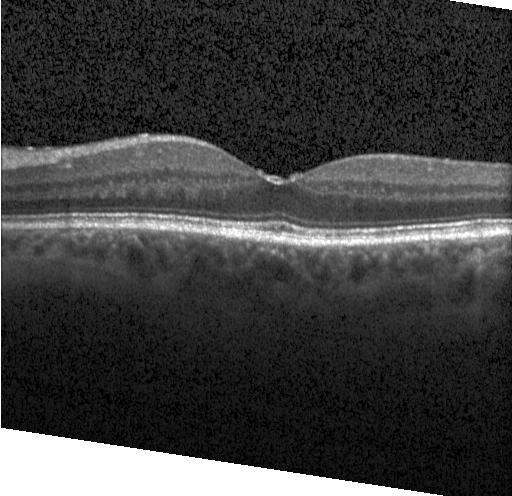
Optical coherence tomography B-scan, spectral-domain OCT, acquired on a Heidelberg Spectralis — Dx: neither choroidal neovascularization, diabetic macular edema, nor drusen.